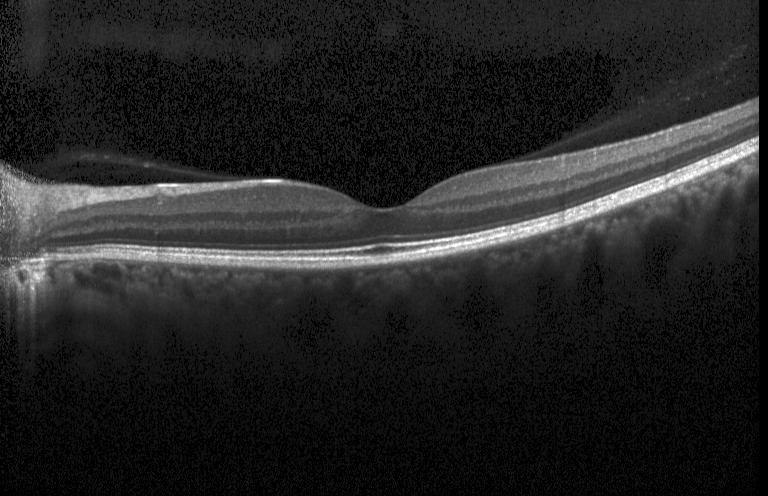

Heidelberg Spectralis. Centered on the fovea. Retinal OCT cross-section. Spectral-domain OCT.
Macular OCT: no choroidal neovascularization, diabetic macular edema, or drusen.